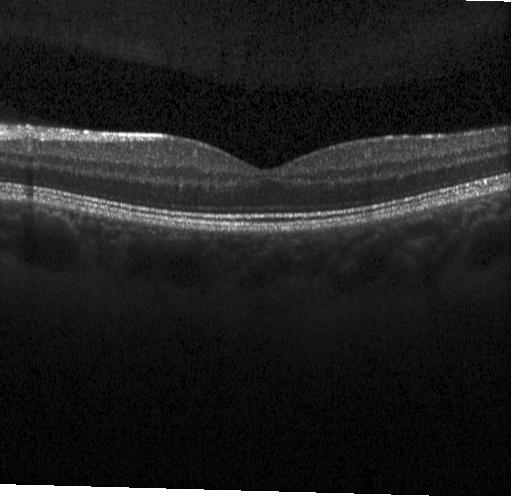

Dx: no CNV, DME, or drusen.